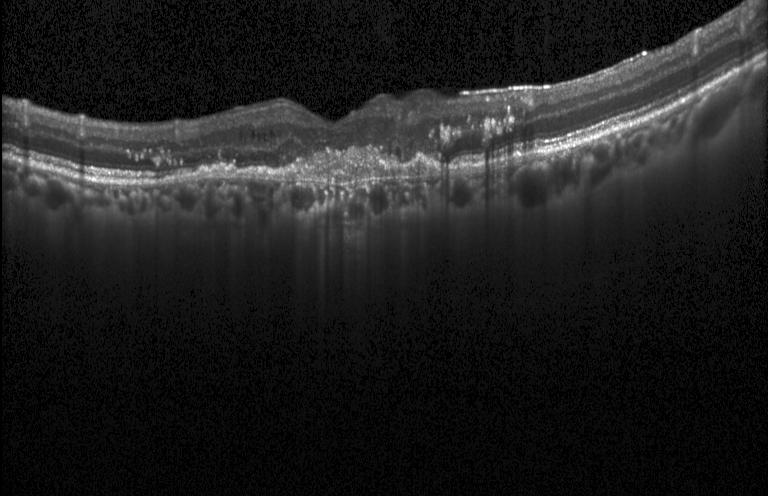
Retinal OCT B-scan · fovea-centered · spectral-domain optical coherence tomography · Heidelberg Spectralis OCT system. Impression: choroidal neovascularization (CNV).